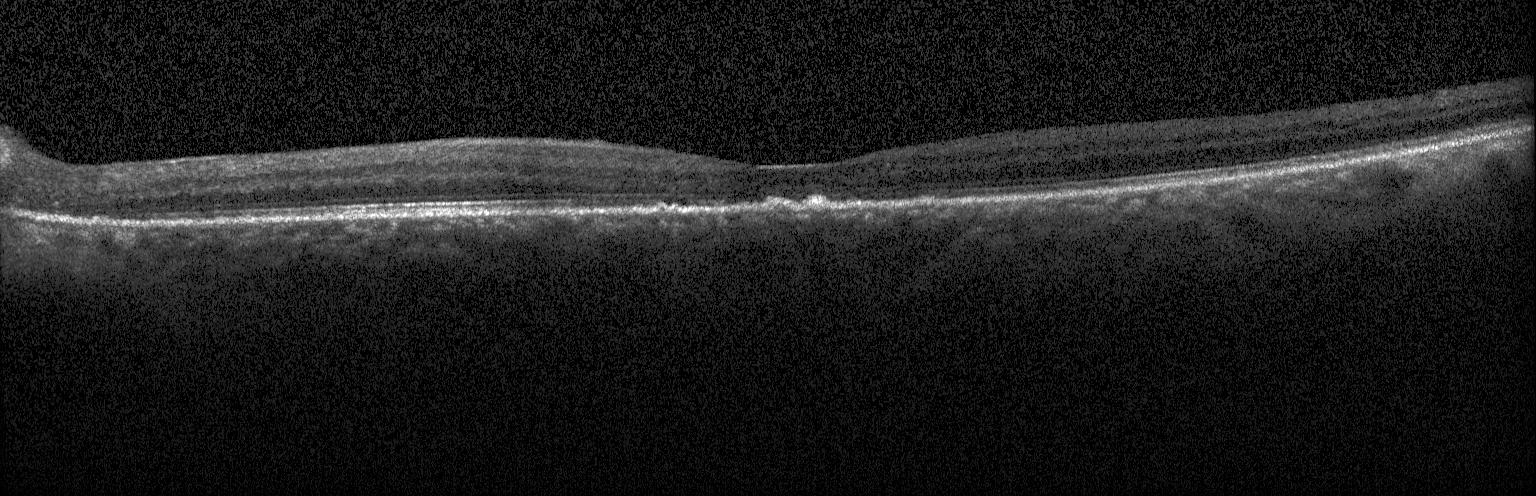

Impression: drusen.